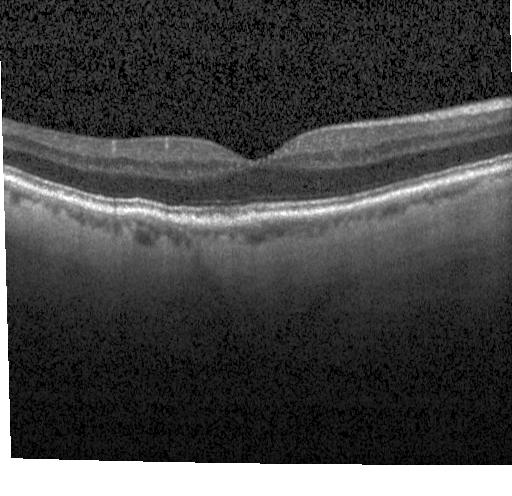 Dx: no evidence of choroidal neovascularization, diabetic macular edema, or drusen.